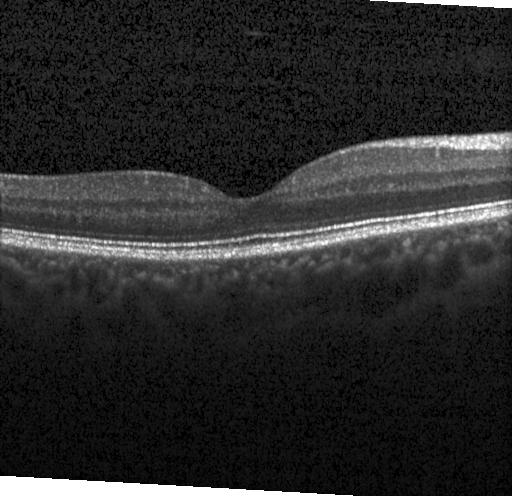

Spectral-domain optical coherence tomography. Fovea-centered. OCT B-scan.
Impression: no evidence of choroidal neovascularization, diabetic macular edema, or drusen.